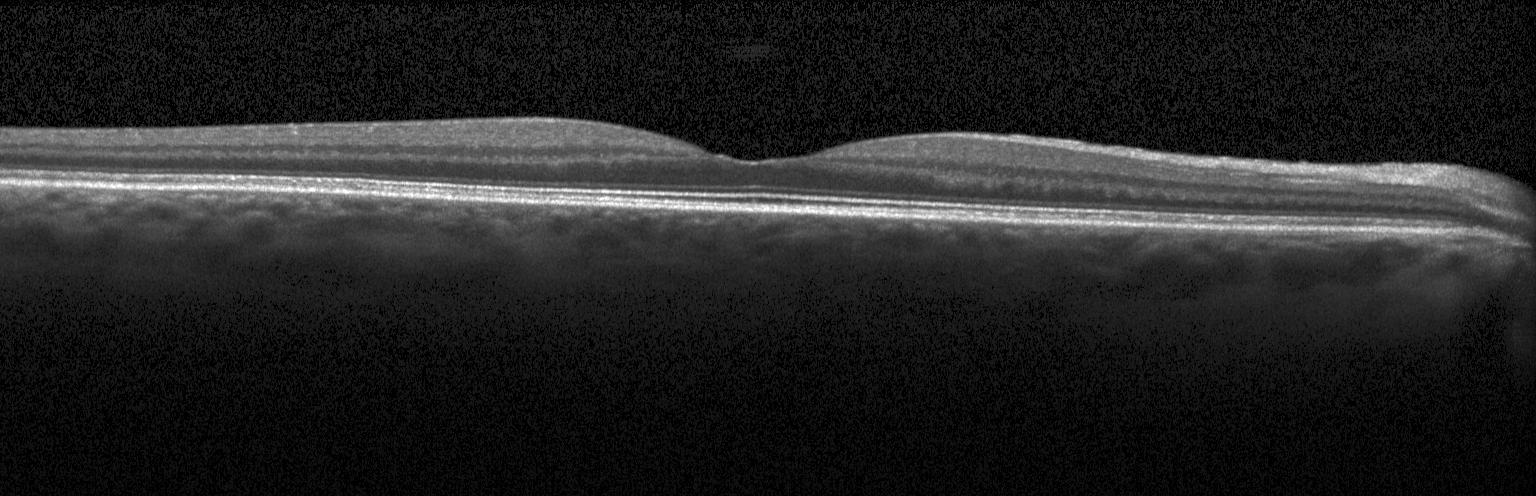 Heidelberg Spectralis OCT system. Retinal OCT B-scan. SD-OCT. Through the macula. Diagnosis: no choroidal neovascularization, no diabetic macular edema, and no drusen.